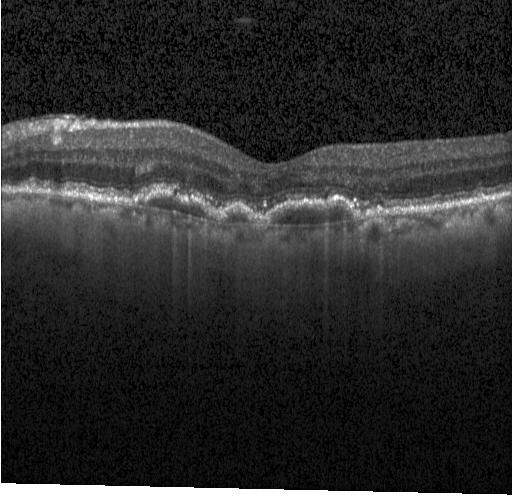 The scan shows choroidal neovascularization.